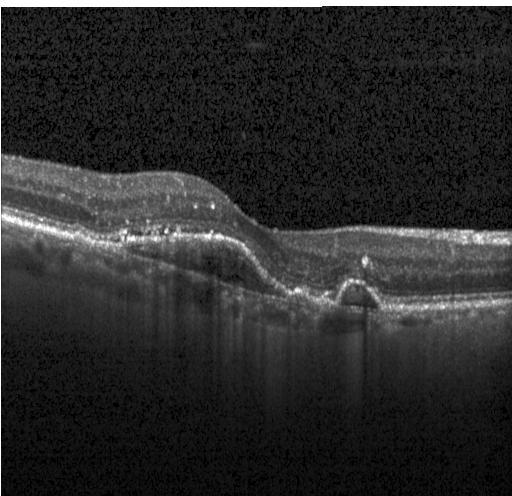

Macular scan; optical coherence tomography scan; acquired on a Heidelberg Spectralis; spectral-domain OCT.
Finding: a choroidal neovascular membrane.